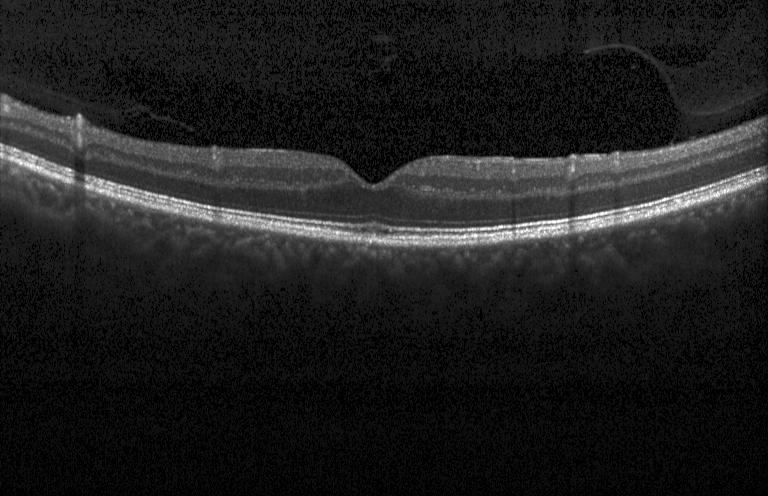
OCT finding: no evidence of choroidal neovascularization, diabetic macular edema, or drusen.